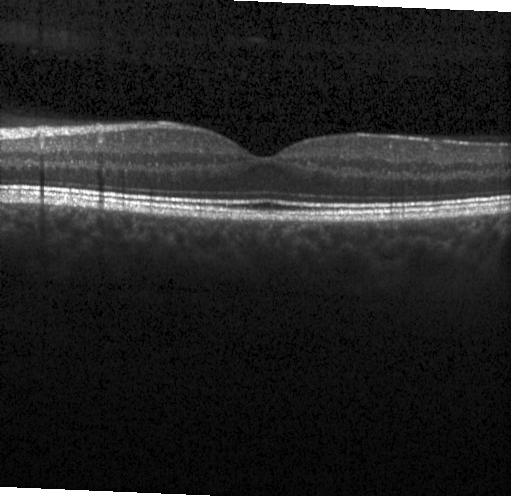

Acquired on a Heidelberg Spectralis; optical coherence tomography scan. Neither CNV, DME, nor drusen.